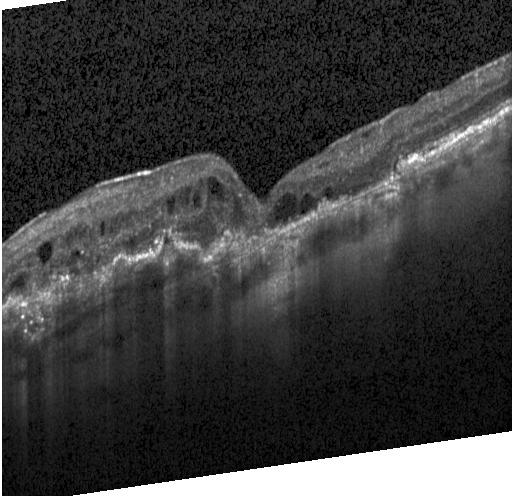 Impression: a choroidal neovascular membrane.